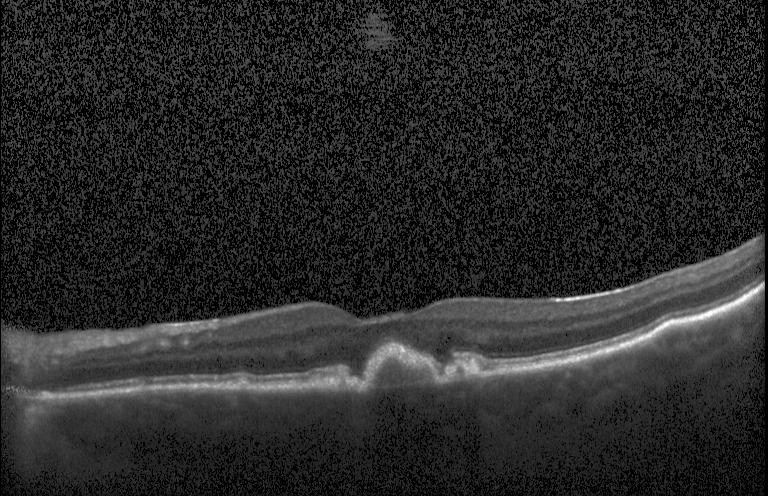
Macular scan; spectral-domain OCT; acquired on a Heidelberg Spectralis; OCT line scan. The scan shows multiple drusen.